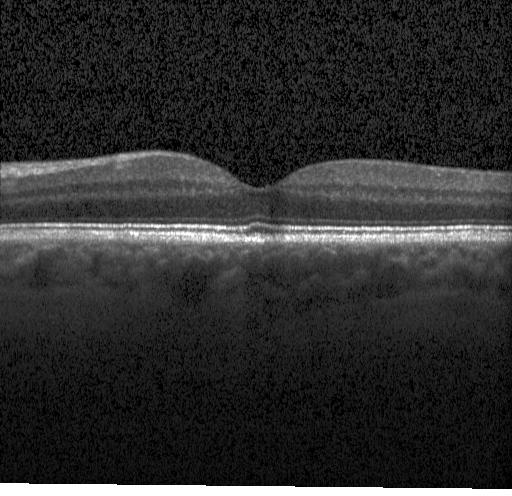 Acquired on a Heidelberg Spectralis, fovea-centered, optical coherence tomography B-scan
The scan shows neither choroidal neovascularization, diabetic macular edema, nor drusen.